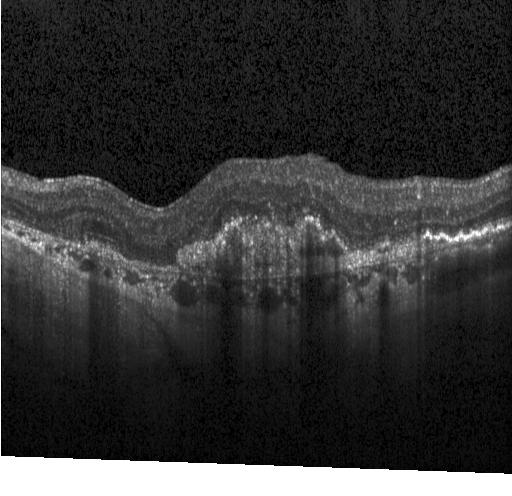 Impression: choroidal neovascularization (CNV).